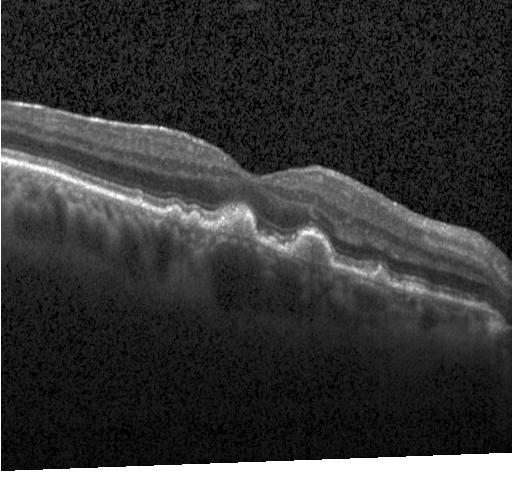
Retinal OCT B-scan. The scan shows multiple drusen.